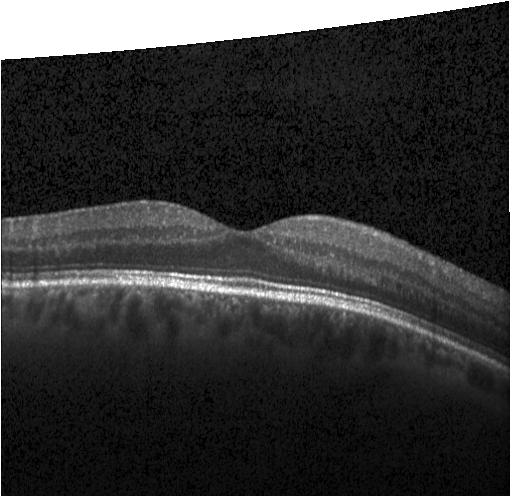
Fovea-centered; OCT B-scan.
The scan shows neither choroidal neovascularization, diabetic macular edema, nor drusen.